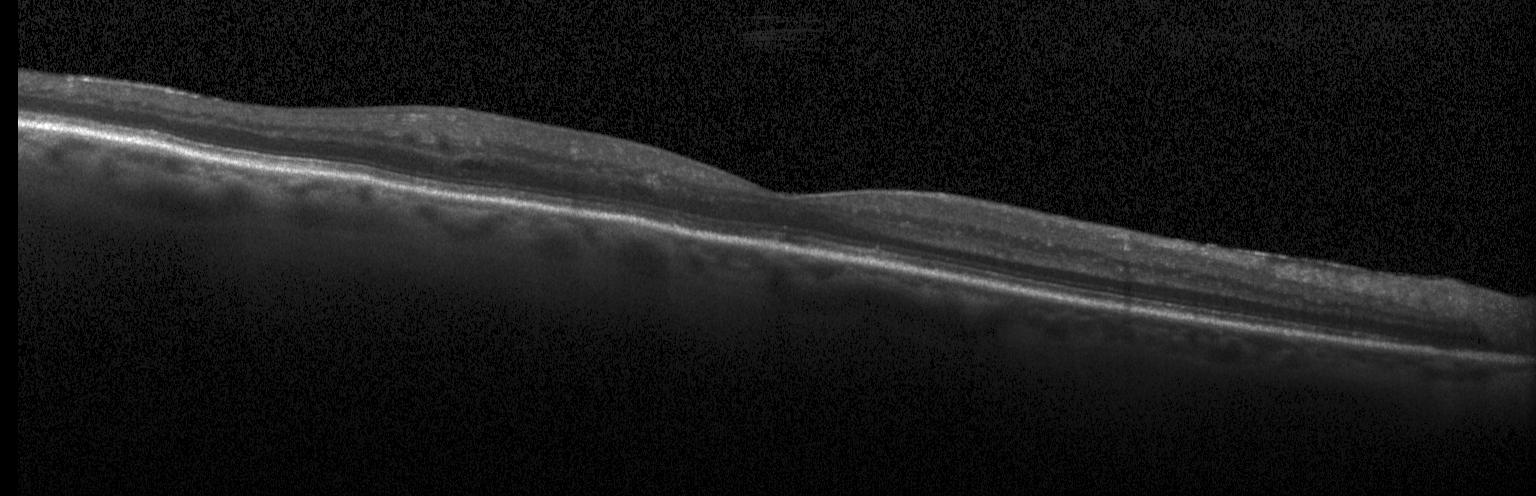 Impression: no choroidal neovascularization, no diabetic macular edema, and no drusen.